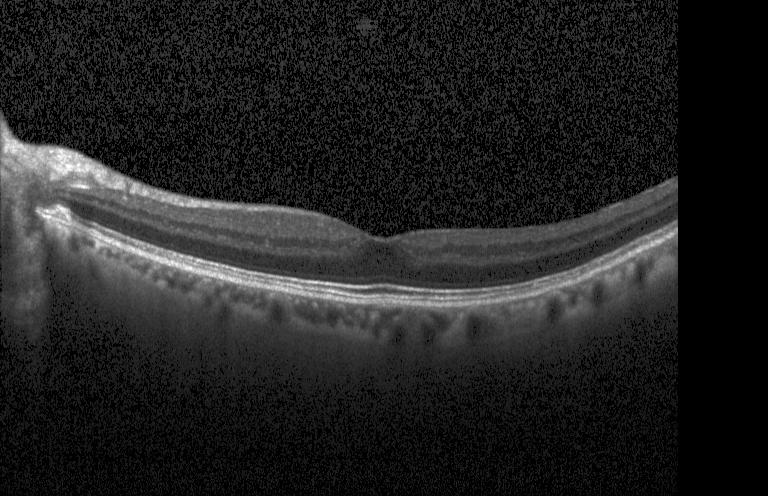

Heidelberg Spectralis OCT system. Macular scan. Retinal OCT cross-section. Spectral-domain OCT. This B-scan demonstrates no evidence of choroidal neovascularization, diabetic macular edema, or drusen.